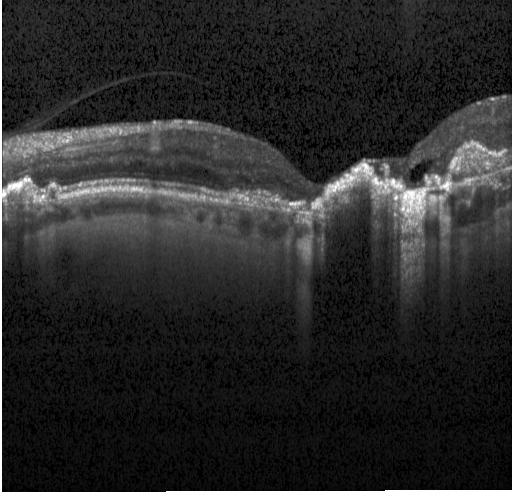 Spectral-domain optical coherence tomography · OCT line scan · Heidelberg Spectralis OCT system · centered on the fovea. CNV.